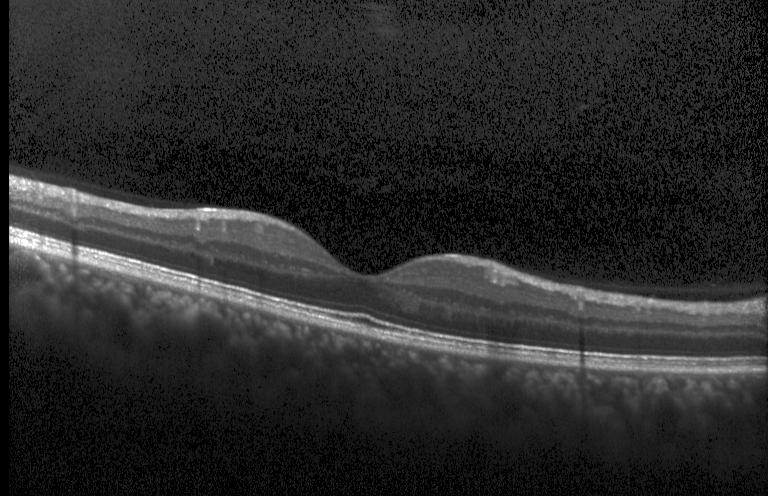
Finding: no choroidal neovascularization, diabetic macular edema, or drusen.